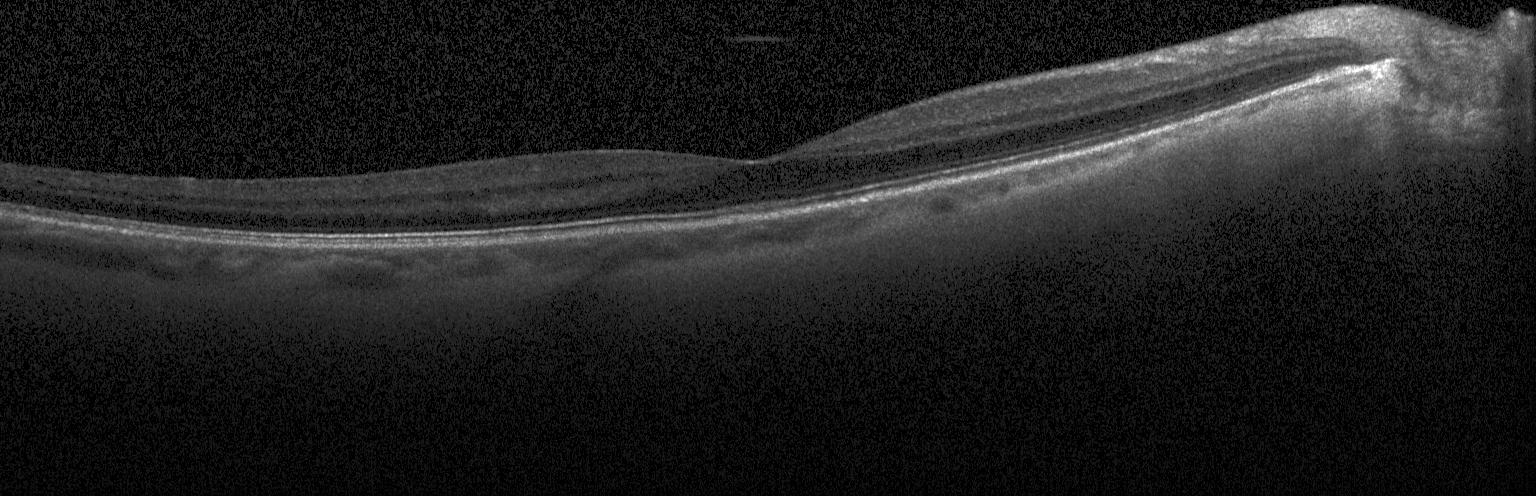 Retinal OCT B-scan · instrument: Heidelberg Spectralis · spectral-domain optical coherence tomography · macular scan — Diagnosis: no CNV, DME, or drusen.